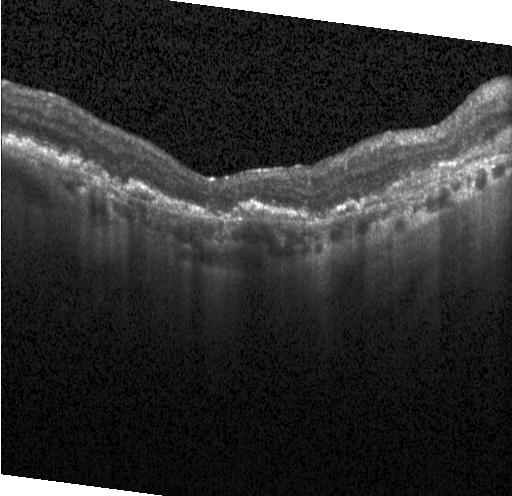
Impression: CNV.